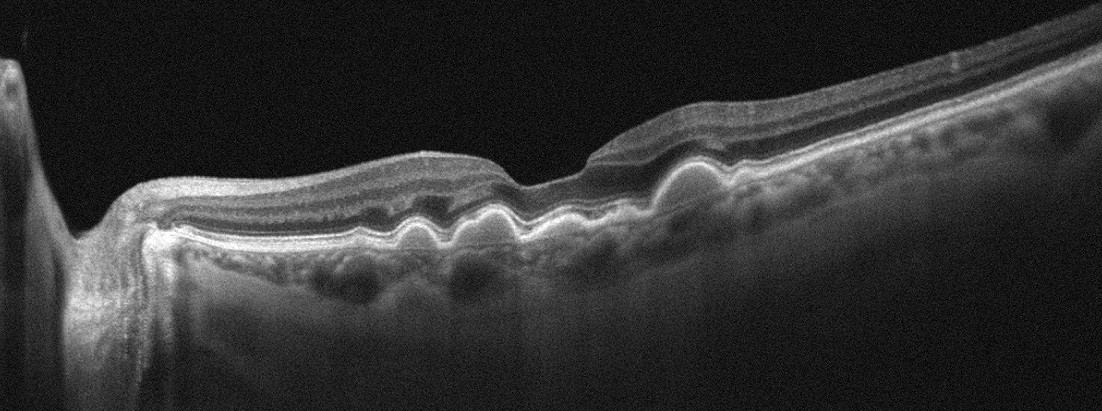

Impression: AMD.